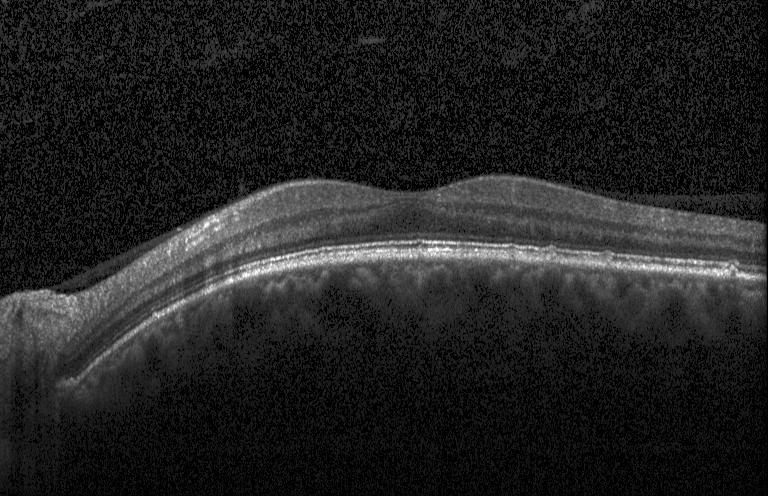

OCT B-scan
Sub-RPE drusenoid deposits.